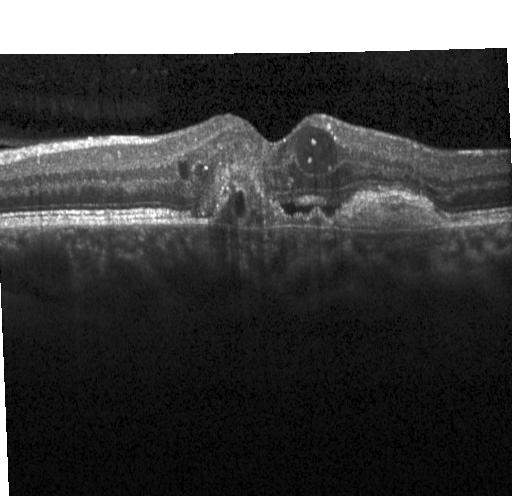

Spectral-domain optical coherence tomography; macular scan; retinal OCT B-scan
OCT finding: a choroidal neovascular membrane.